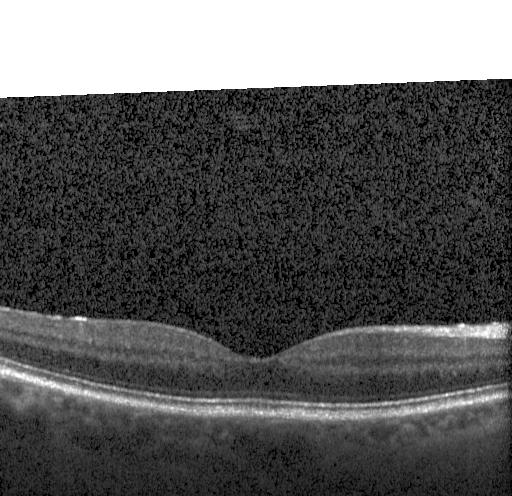
Optical coherence tomography B-scan. SD-OCT. Diagnosis: neither choroidal neovascularization, diabetic macular edema, nor drusen.